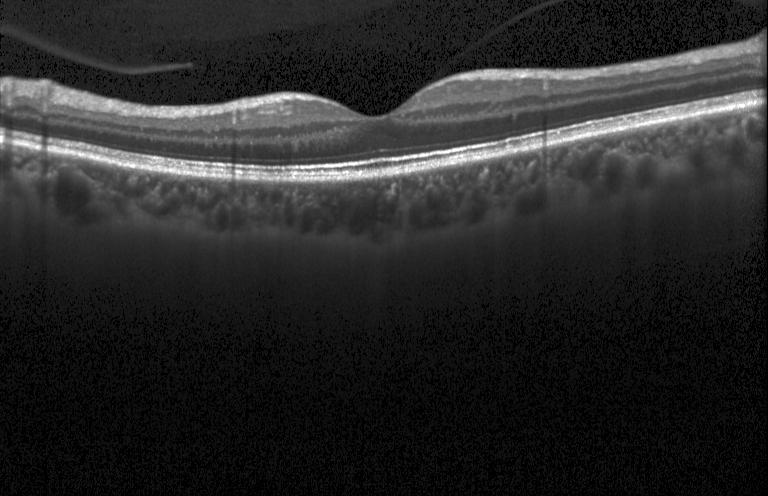 OCT line scan.
Assessment: no evidence of choroidal neovascularization, diabetic macular edema, or drusen.